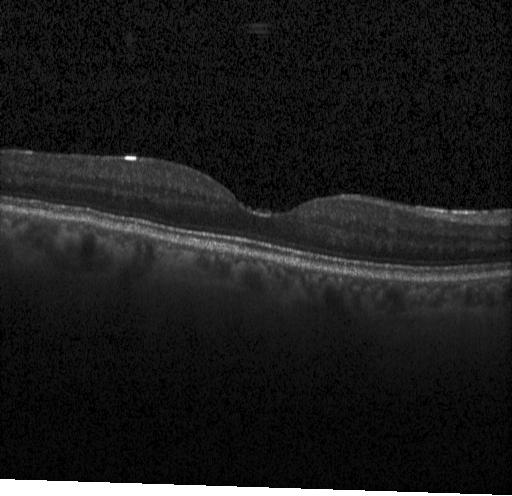
Fovea-centered. Retinal OCT cross-section. SD-OCT. Acquired on a Heidelberg Spectralis. Impression: no CNV, no DME, and no drusen.